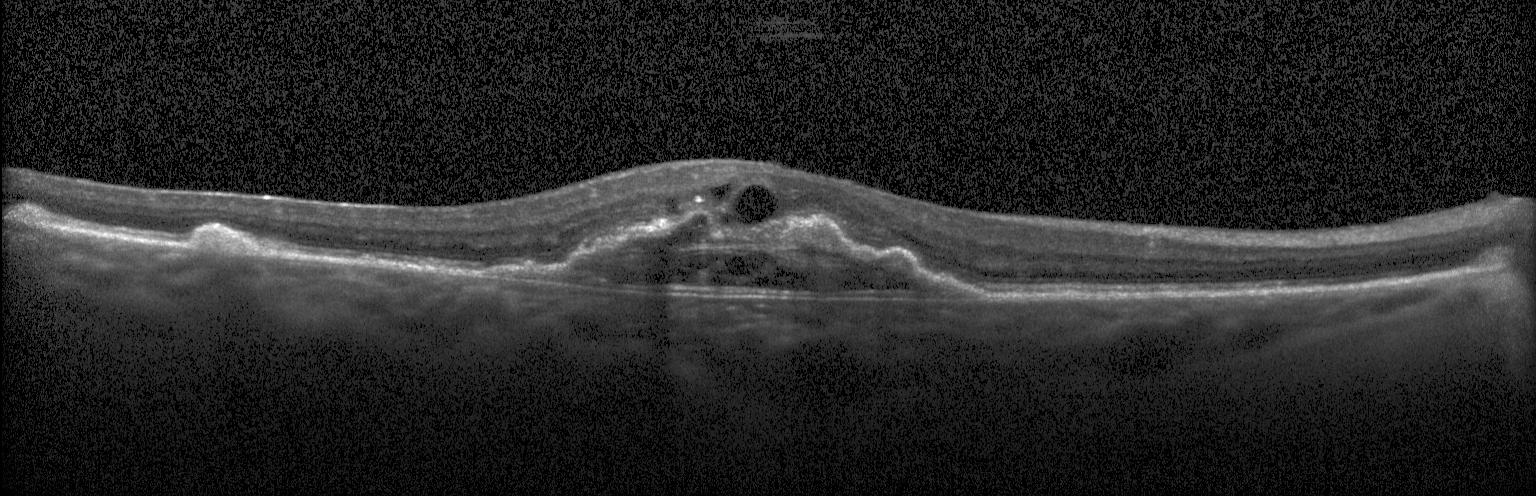
Assessment: a choroidal neovascular membrane.